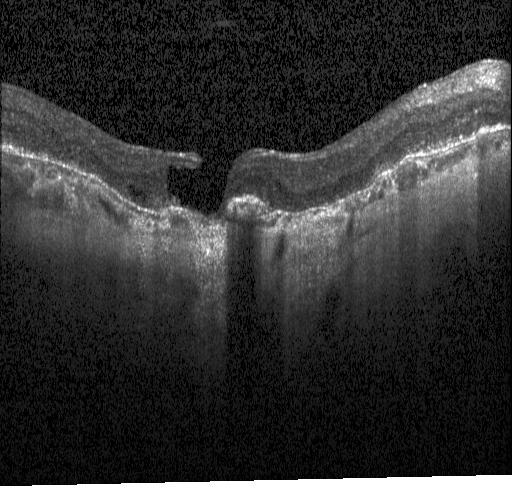 Diagnosis: a choroidal neovascular membrane.